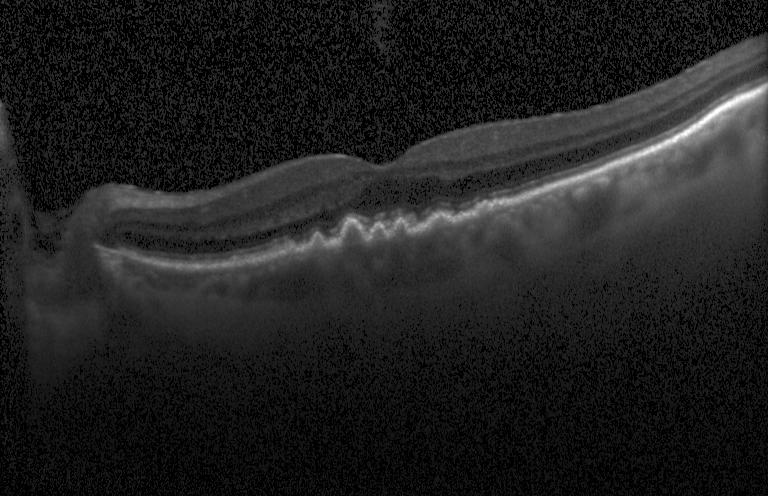
Impression: sub-RPE drusenoid deposits.